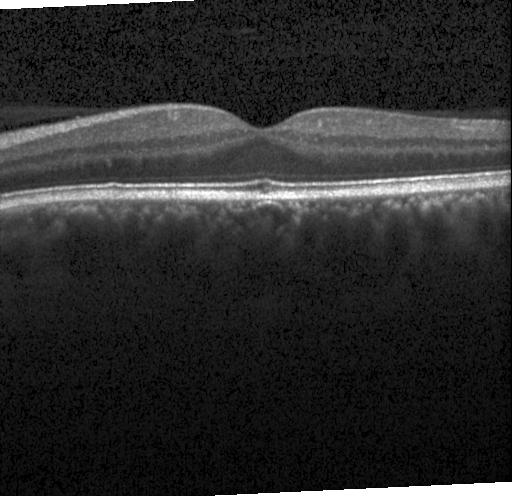

Heidelberg Spectralis OCT system. OCT B-scan. Spectral-domain OCT. Fovea-centered.
This B-scan demonstrates no CNV, no DME, and no drusen.